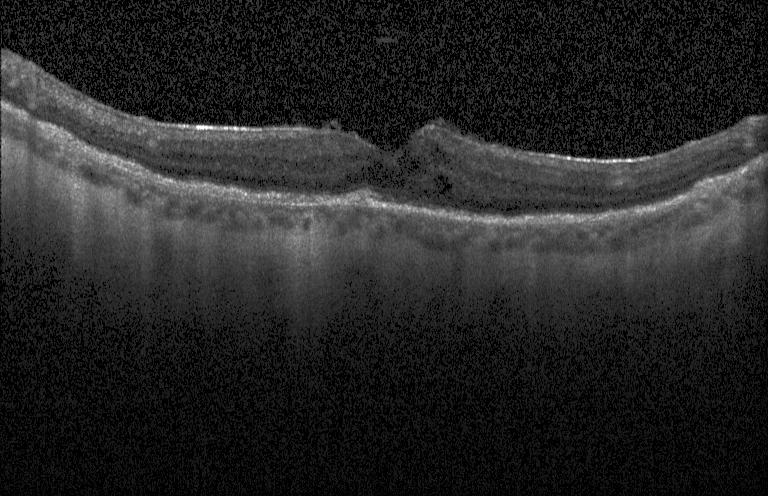
Centered on the fovea, optical coherence tomography B-scan, spectral-domain optical coherence tomography.
Impression: diabetic macular edema.